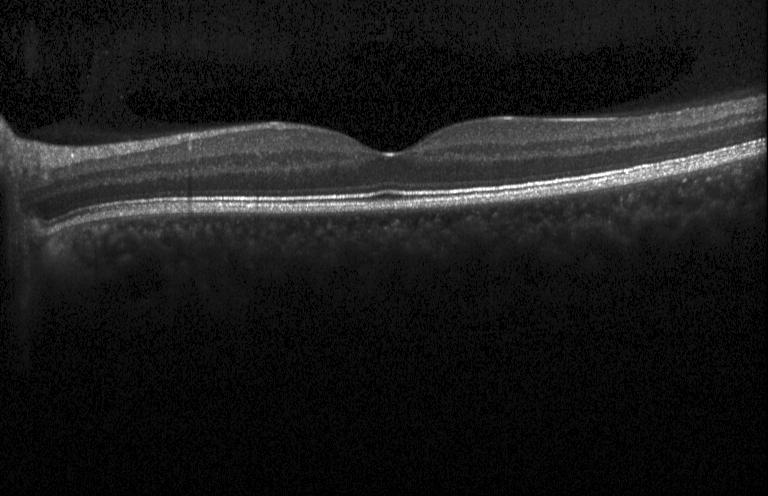
Heidelberg Spectralis. Retinal OCT cross-section — This B-scan demonstrates no evidence of choroidal neovascularization, diabetic macular edema, or drusen.